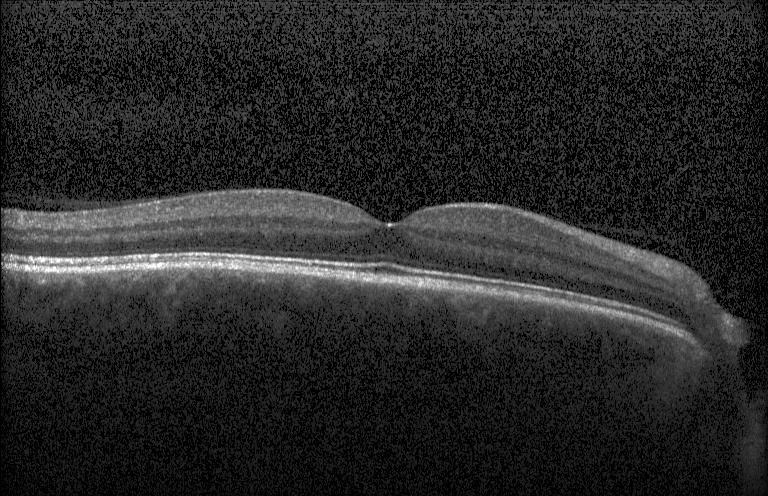 Macular OCT demonstrating neither CNV, DME, nor drusen.